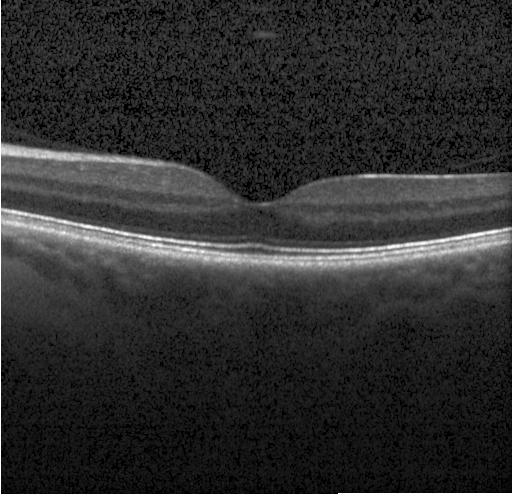

Retinal OCT cross-section; spectral-domain optical coherence tomography; Heidelberg Spectralis
This B-scan demonstrates no choroidal neovascularization, no diabetic macular edema, and no drusen.